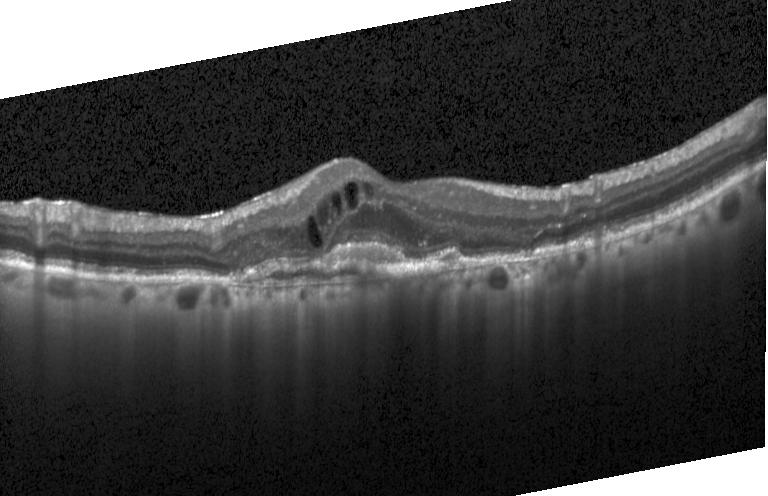 Acquired on a Heidelberg Spectralis · spectral-domain OCT · OCT B-scan. Finding: choroidal neovascularization (CNV).